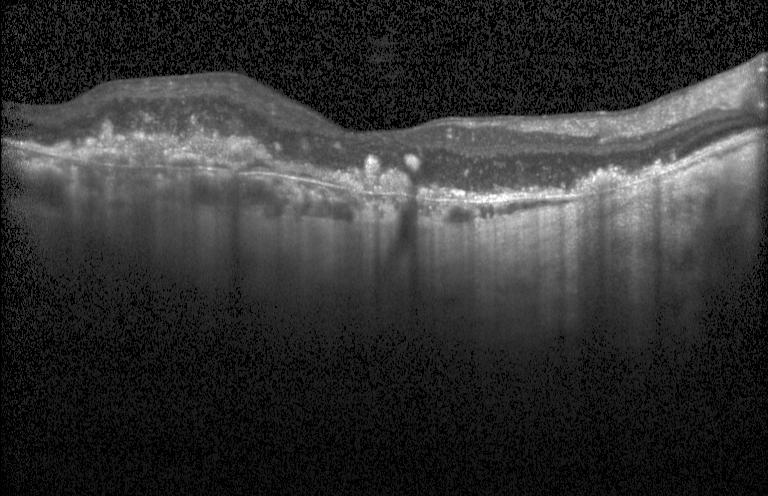
OCT finding: a choroidal neovascular membrane.